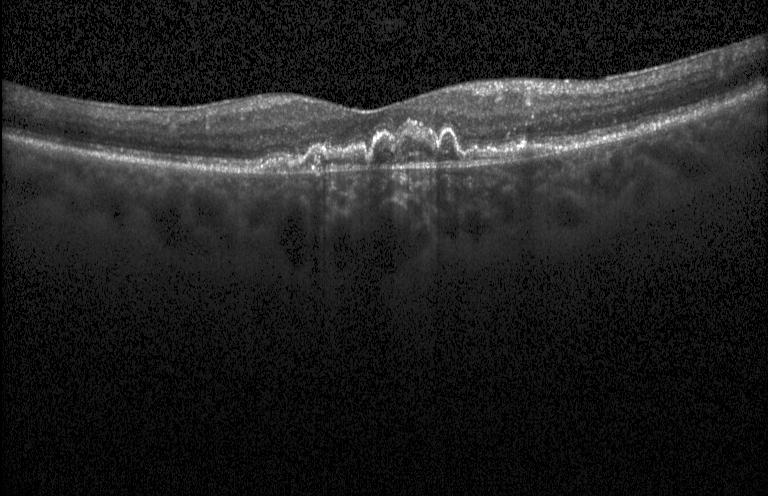
Retinal OCT cross-section showing a choroidal neovascular membrane.